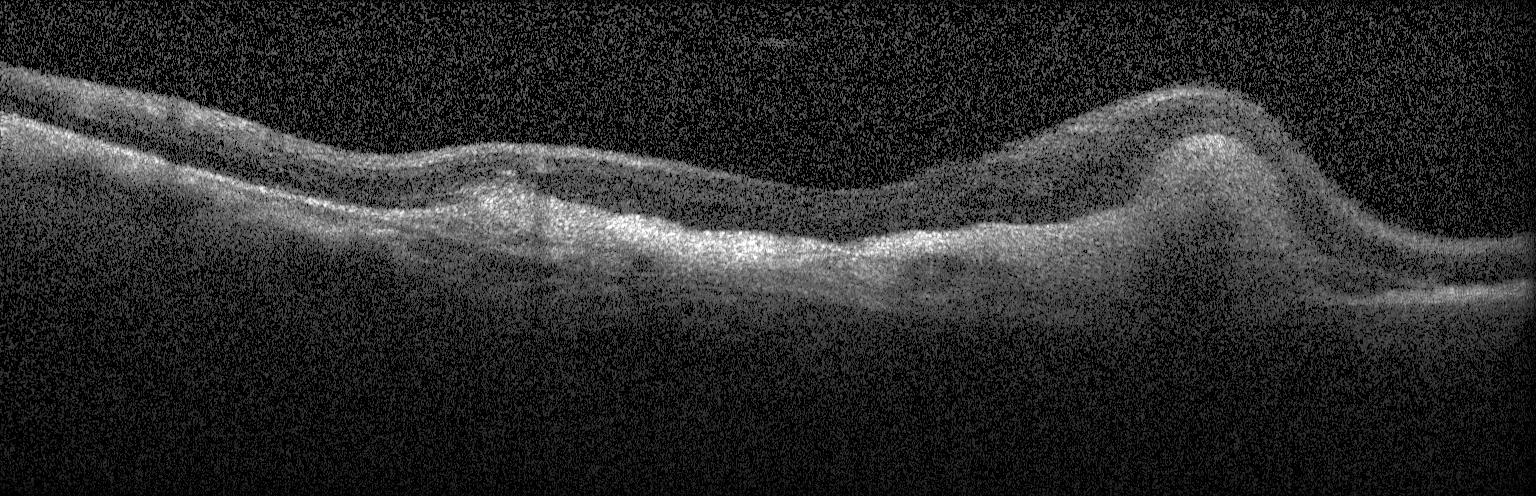
Optical coherence tomography scan
This B-scan demonstrates a choroidal neovascular membrane.